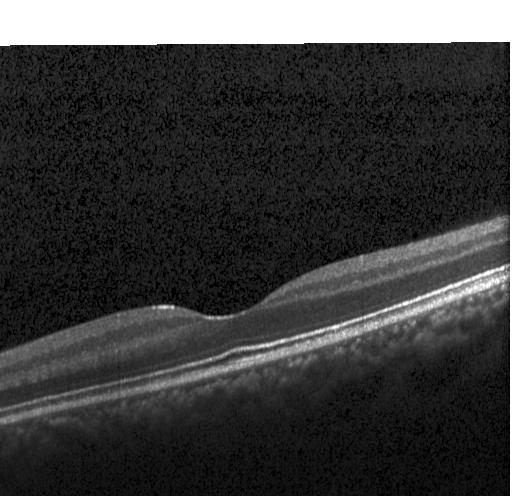
Finding: neither choroidal neovascularization, diabetic macular edema, nor drusen.